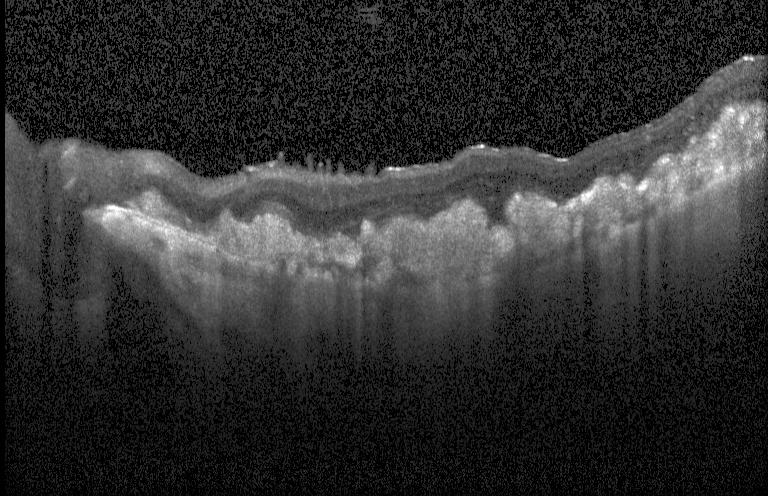

Fovea-centered · SD-OCT · OCT B-scan. OCT finding: a choroidal neovascular membrane.